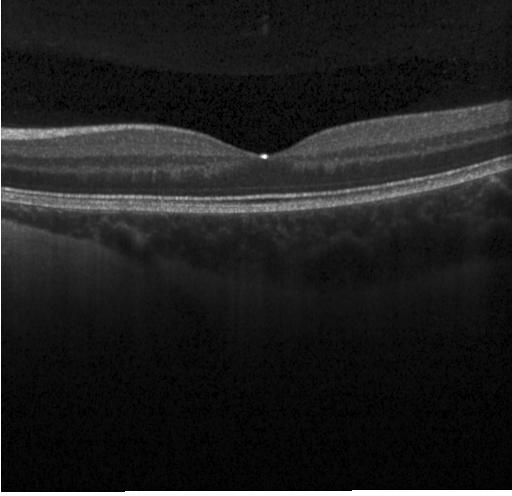

OCT B-scan.
The scan shows no evidence of CNV, DME, or drusen.